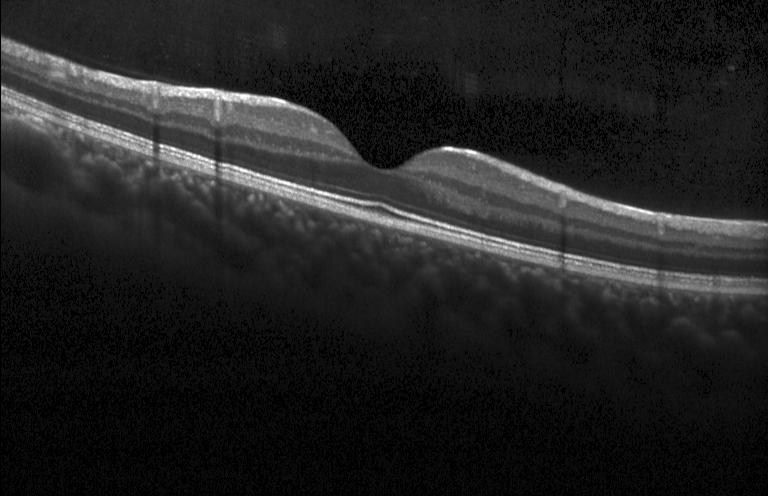
SD-OCT, retinal OCT cross-section — Dx: no evidence of CNV, DME, or drusen.